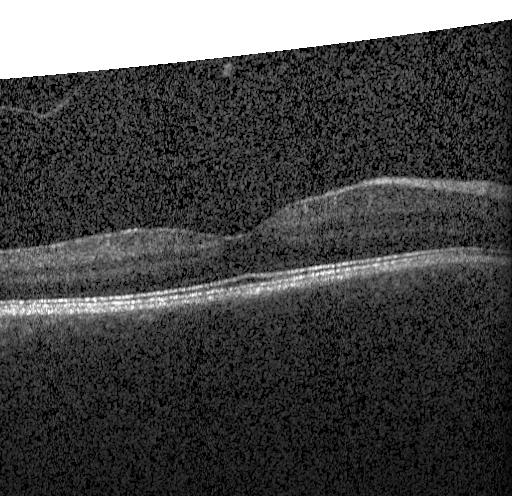
Impression: neither choroidal neovascularization, diabetic macular edema, nor drusen.